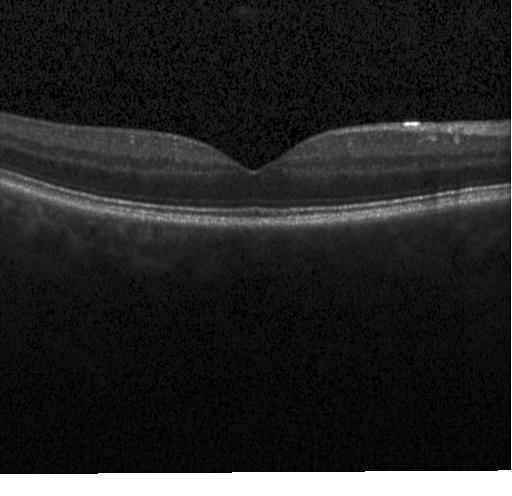 Horizontal scan through the fovea. Instrument: Heidelberg Spectralis. OCT B-scan. SD-OCT.
No choroidal neovascularization, diabetic macular edema, or drusen.